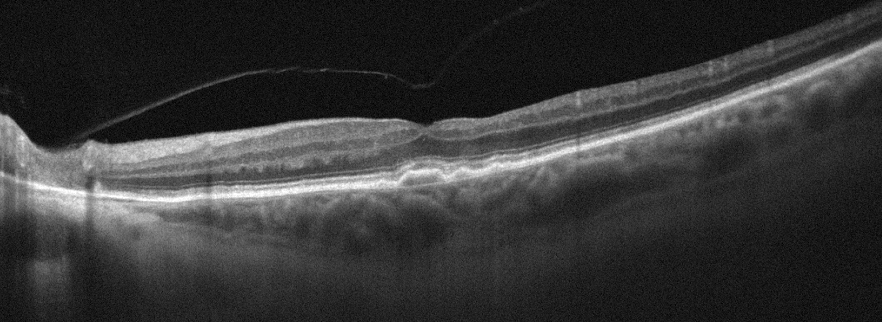

Left eye; optical coherence tomography scan.
Diagnosis: AMD.